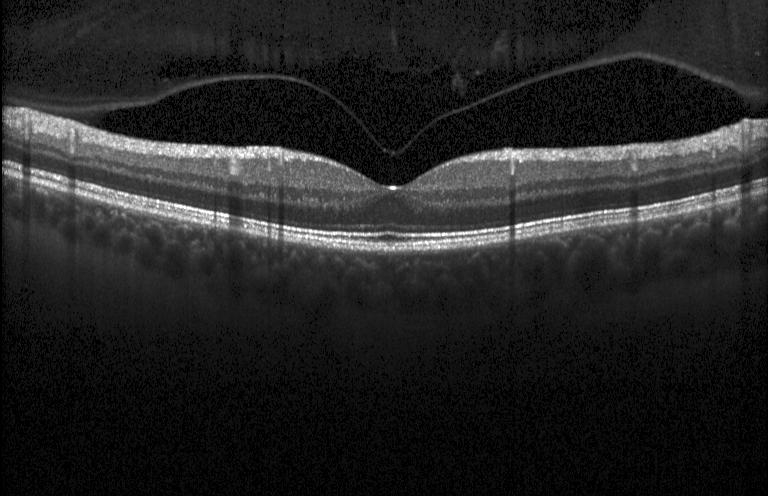
Centered on the fovea; OCT B-scan; spectral-domain OCT; Heidelberg Spectralis OCT system. This B-scan demonstrates neither choroidal neovascularization, diabetic macular edema, nor drusen.